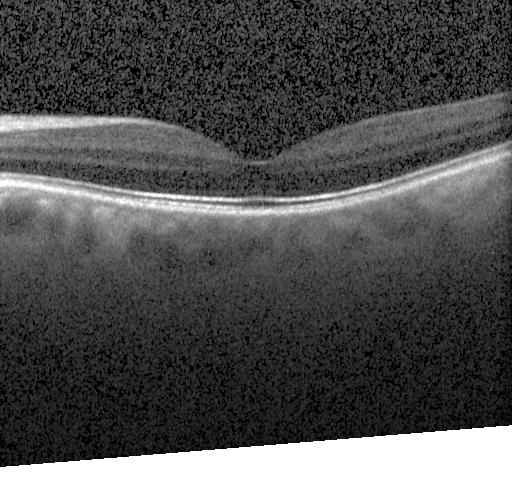
Instrument: Heidelberg Spectralis · retinal OCT B-scan · spectral-domain OCT · macular scan
Finding: neither choroidal neovascularization, diabetic macular edema, nor drusen.